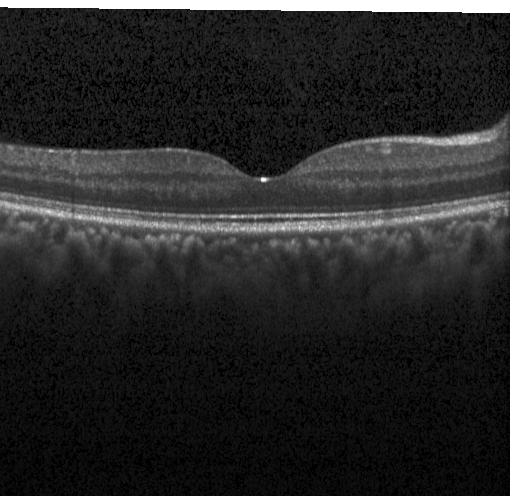
Heidelberg Spectralis OCT system. Centered on the fovea. Retinal OCT cross-section.
OCT finding: neither CNV, DME, nor drusen.